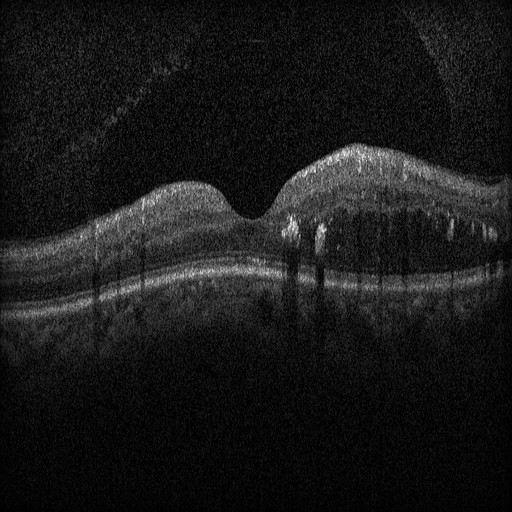 Impression: diabetic macular edema.